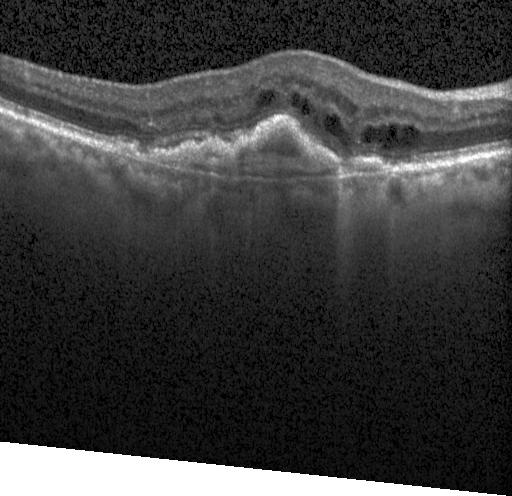
Impression: CNV.